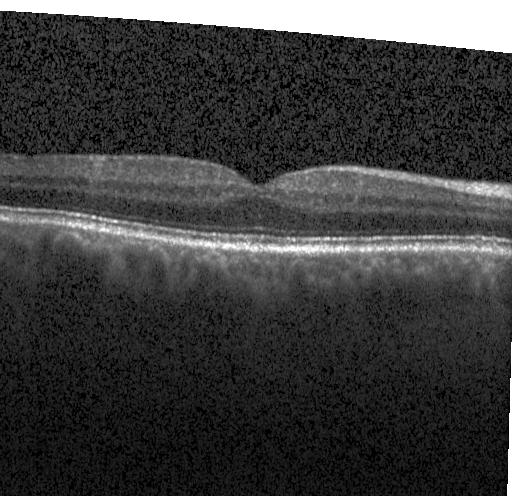
SD-OCT, retinal OCT cross-section, Heidelberg Spectralis, macular scan
Macular OCT: no CNV, DME, or drusen.